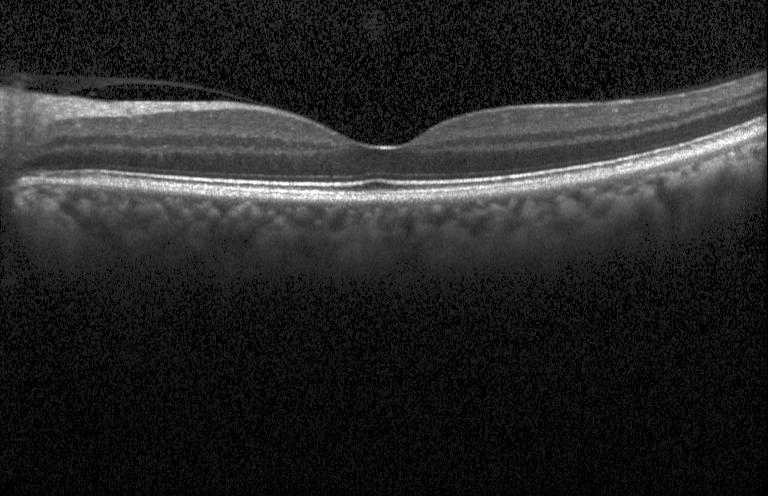
Through the macula. Optical coherence tomography B-scan. Heidelberg Spectralis OCT system. SD-OCT. Dx: no evidence of choroidal neovascularization, diabetic macular edema, or drusen.